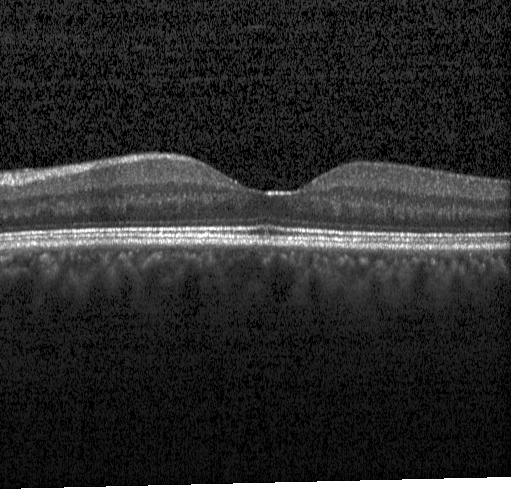

Instrument: Heidelberg Spectralis · optical coherence tomography scan.
Impression: neither choroidal neovascularization, diabetic macular edema, nor drusen.